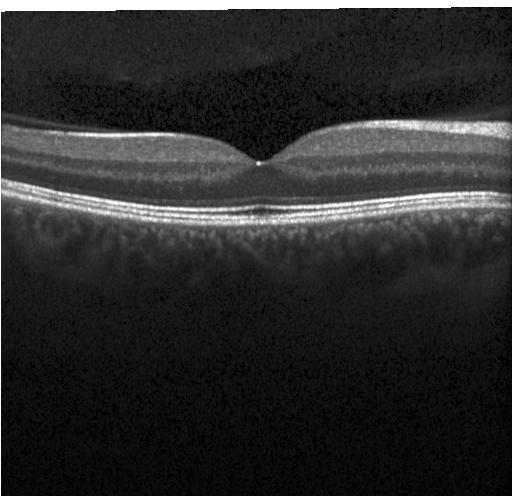

SD-OCT · acquired on a Heidelberg Spectralis · centered on the fovea · optical coherence tomography scan — Diagnosis: neither choroidal neovascularization, diabetic macular edema, nor drusen.